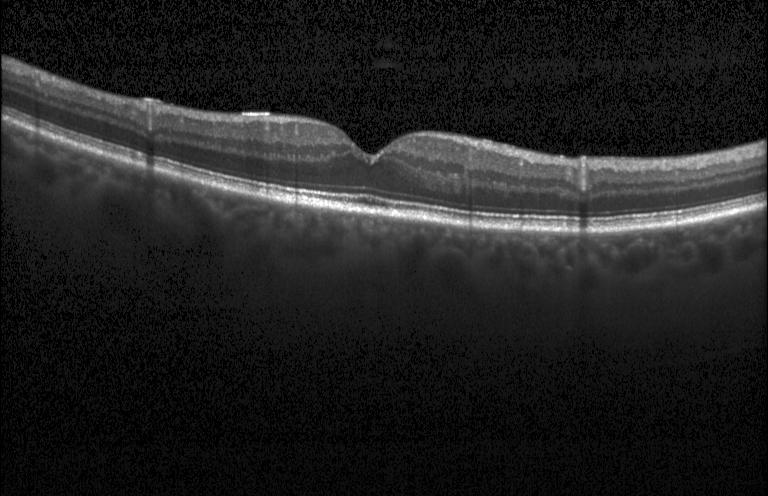

SD-OCT. Optical coherence tomography B-scan. Finding: no choroidal neovascularization, no diabetic macular edema, and no drusen.